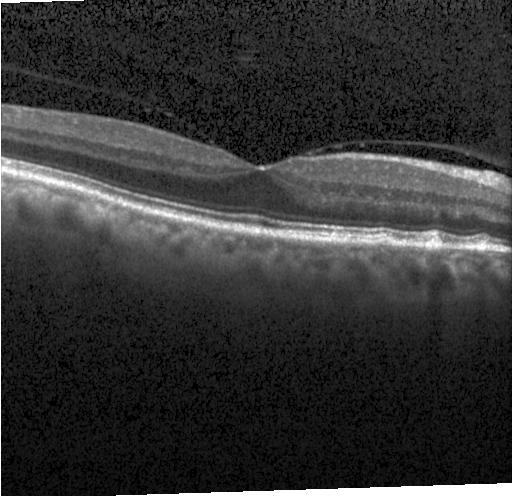 Finding: sub-RPE drusenoid deposits.